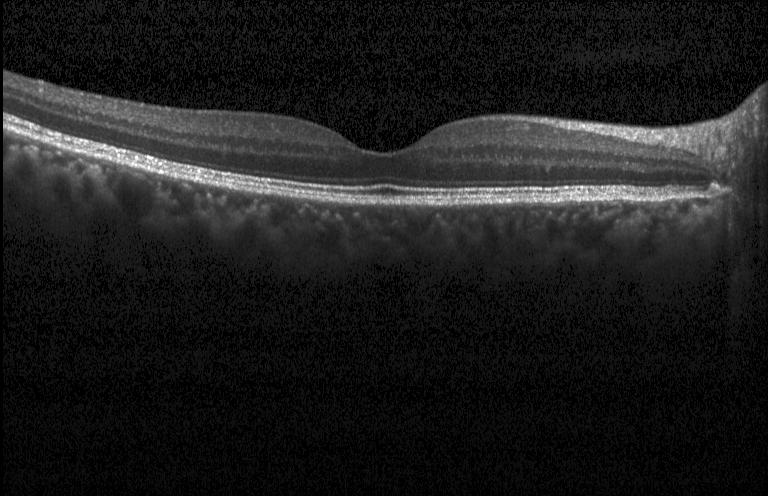 Macular OCT demonstrating no evidence of choroidal neovascularization, diabetic macular edema, or drusen.